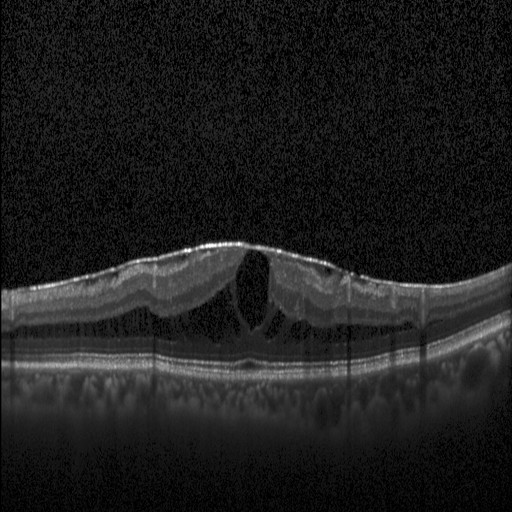
Instrument: Heidelberg Spectralis · retinal OCT B-scan · fovea-centered · spectral-domain optical coherence tomography
Impression: diabetic macular edema (DME).